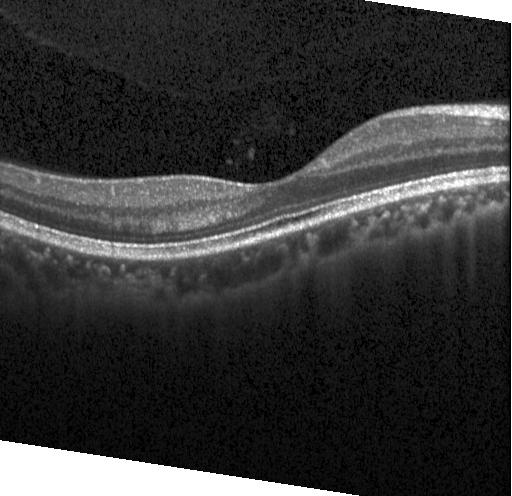
Heidelberg Spectralis · spectral-domain OCT · retinal OCT cross-section.
Diagnosis: no choroidal neovascularization, diabetic macular edema, or drusen.